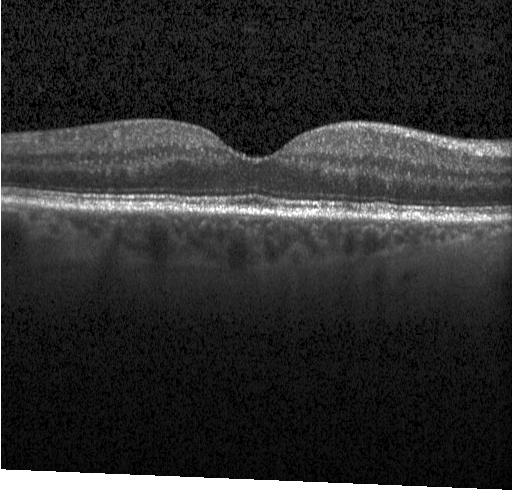
Heidelberg Spectralis OCT system. Retinal OCT cross-section — Assessment: no evidence of choroidal neovascularization, diabetic macular edema, or drusen.